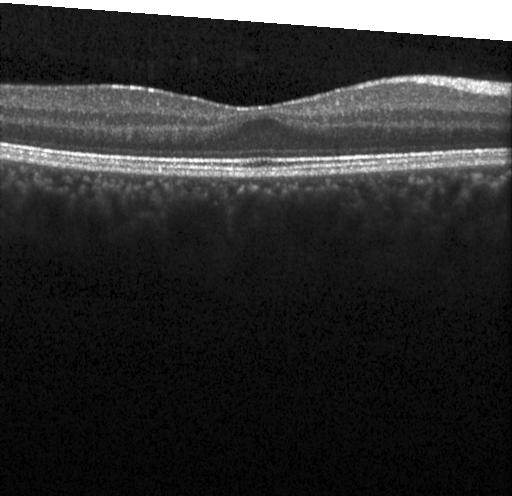 Optical coherence tomography B-scan.
Dx: neither CNV, DME, nor drusen.